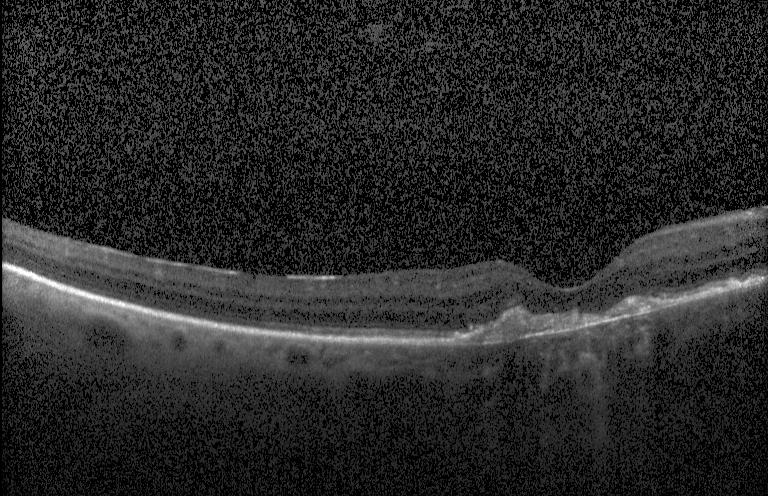

Finding: choroidal neovascularization (CNV).